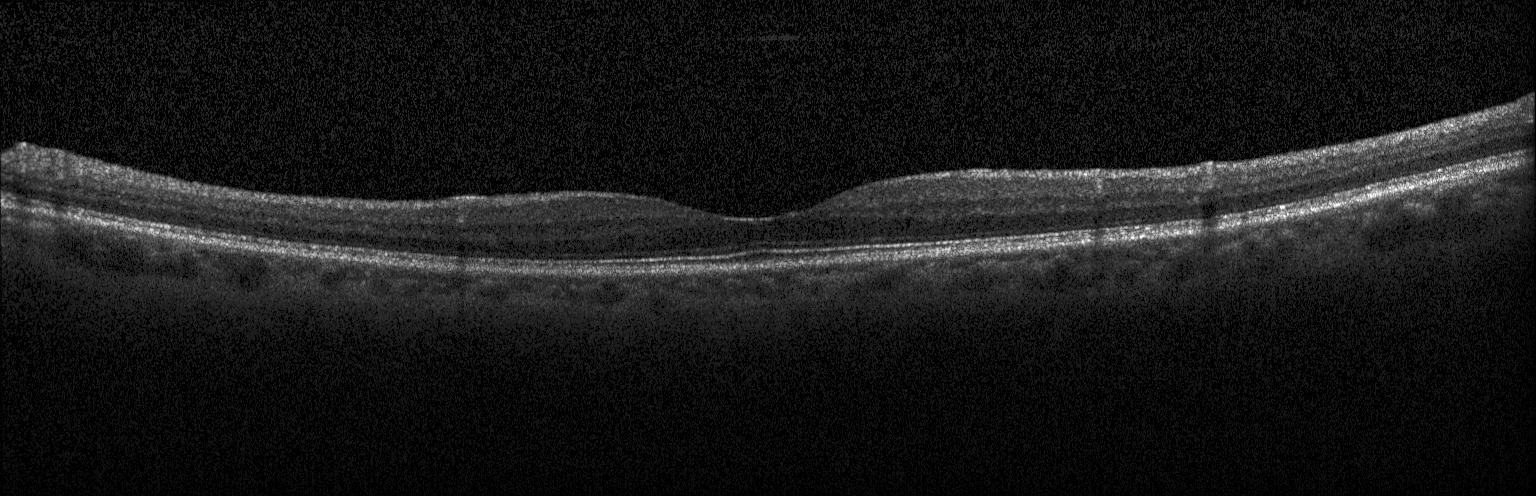
Diagnosis: no choroidal neovascularization, diabetic macular edema, or drusen.